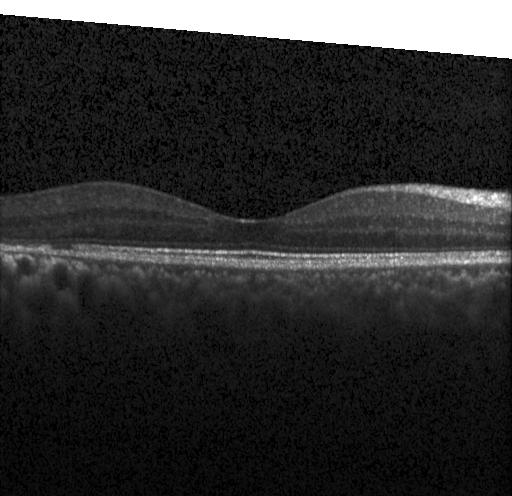

Spectral-domain OCT B-scan: no evidence of choroidal neovascularization, diabetic macular edema, or drusen.